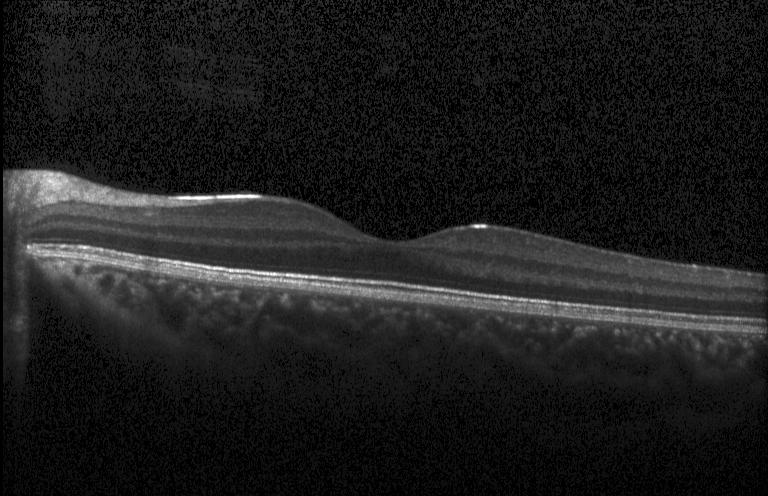
OCT scan showing neither choroidal neovascularization, diabetic macular edema, nor drusen.